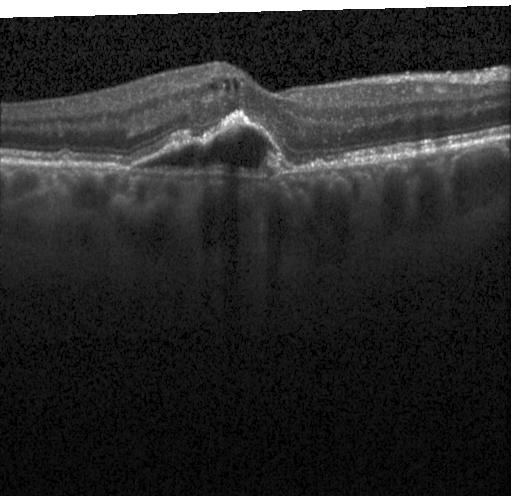

OCT B-scan; spectral-domain OCT.
Finding: a choroidal neovascular membrane.